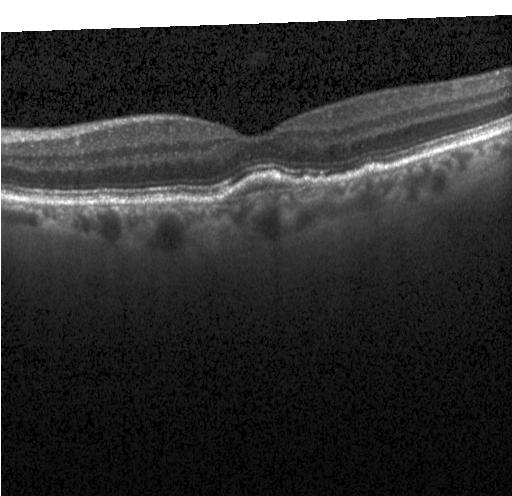

Acquired on a Heidelberg Spectralis; SD-OCT; optical coherence tomography B-scan; centered on the fovea — Dx: a choroidal neovascular membrane.